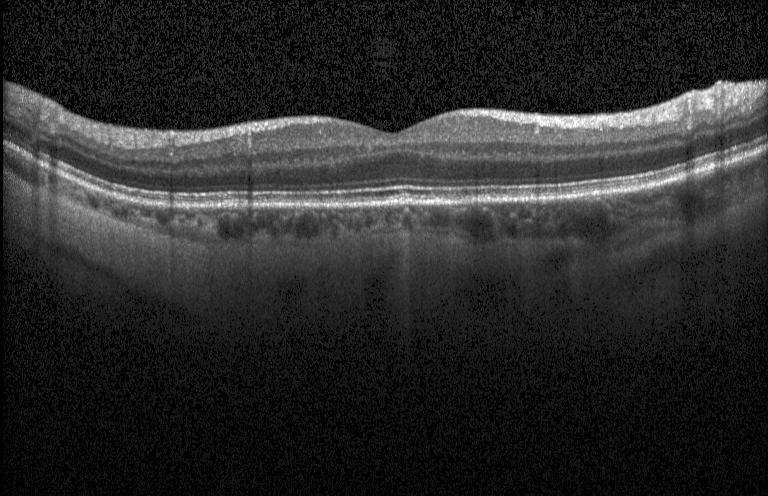 Optical coherence tomography scan.
Finding: no choroidal neovascularization, no diabetic macular edema, and no drusen.